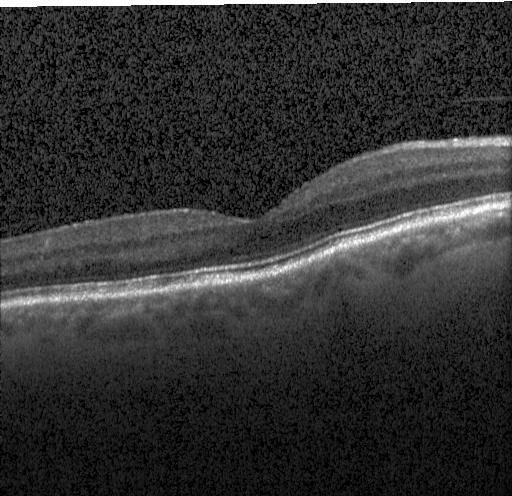 The scan shows no CNV, no DME, and no drusen.